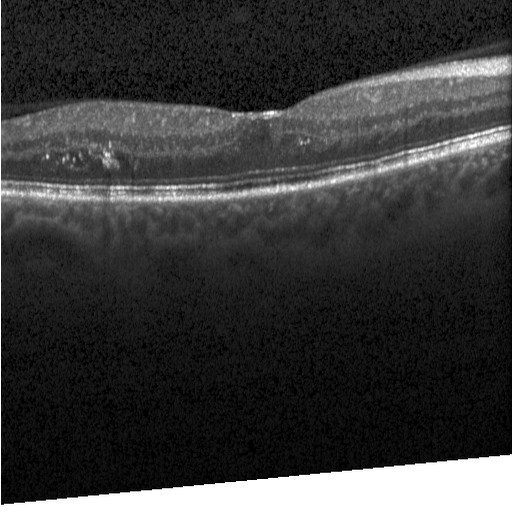

Through the macula, spectral-domain optical coherence tomography, OCT B-scan, instrument: Heidelberg Spectralis — Diabetic macular edema (DME).